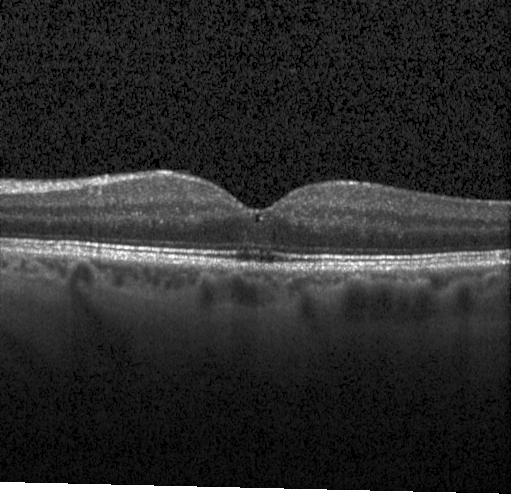
Retinal OCT cross-section. Heidelberg Spectralis
No choroidal neovascularization, diabetic macular edema, or drusen.